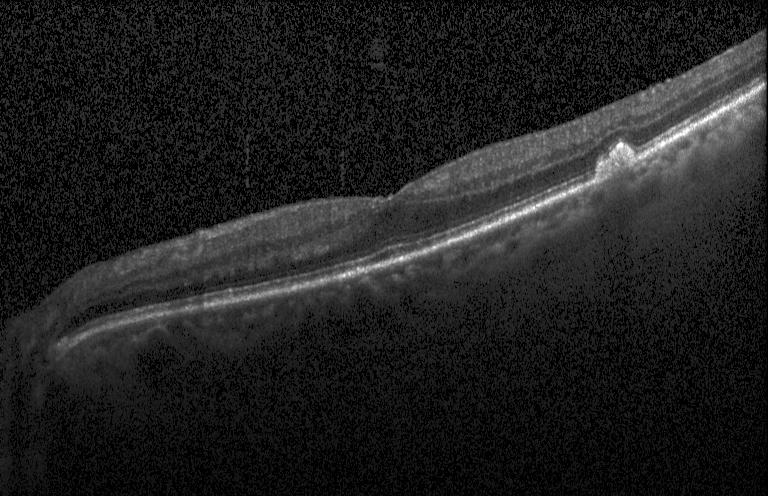

Finding: multiple drusen.